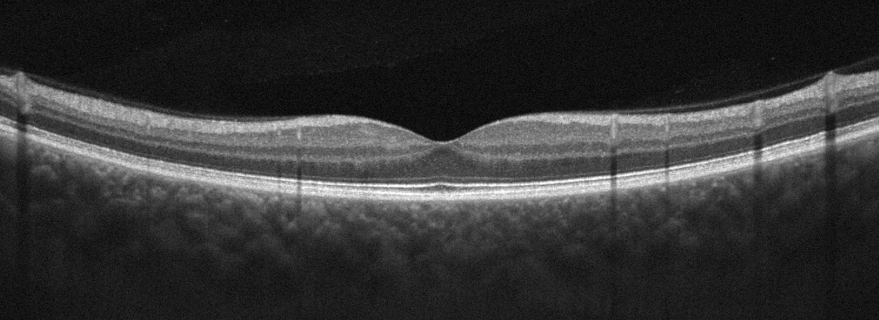 Optovue Avanti RTVue XR, macular scan, retinal OCT cross-section — Diagnosis: no AMD, DME, ERM, RAO, RVO, or VID.